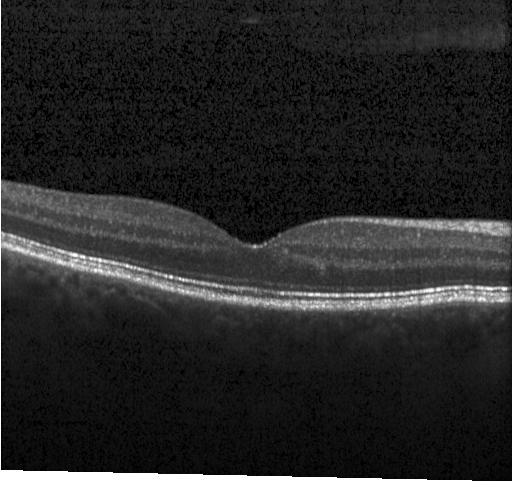 Heidelberg Spectralis OCT system. Optical coherence tomography scan. Spectral-domain optical coherence tomography.
The scan shows no choroidal neovascularization, diabetic macular edema, or drusen.